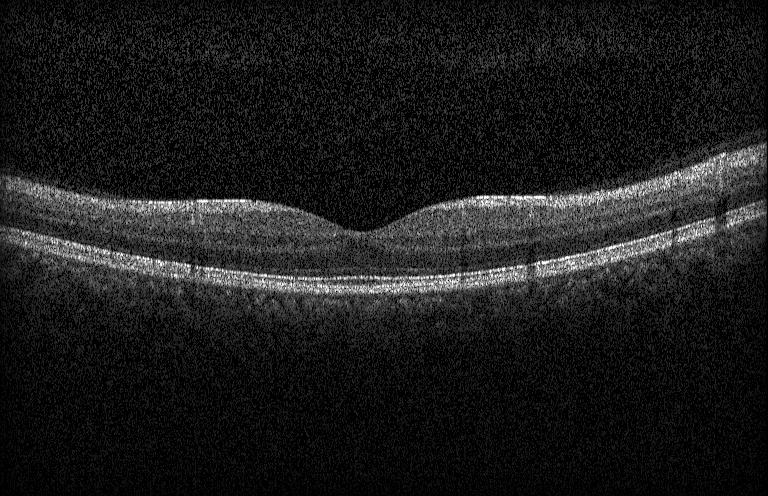 Finding: neither choroidal neovascularization, diabetic macular edema, nor drusen.